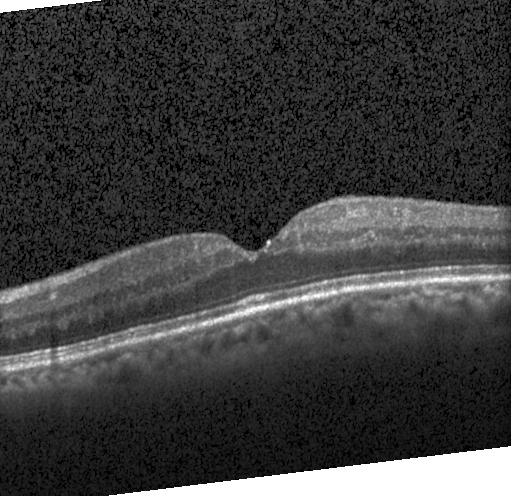 Horizontal scan through the fovea · retinal OCT cross-section · acquired on a Heidelberg Spectralis · spectral-domain OCT
OCT finding: no choroidal neovascularization, no diabetic macular edema, and no drusen.